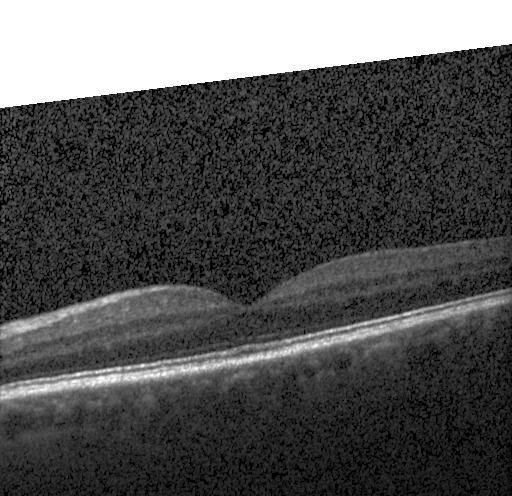

OCT B-scan · horizontal scan through the fovea · spectral-domain optical coherence tomography · acquired on a Heidelberg Spectralis.
Assessment: no evidence of choroidal neovascularization, diabetic macular edema, or drusen.